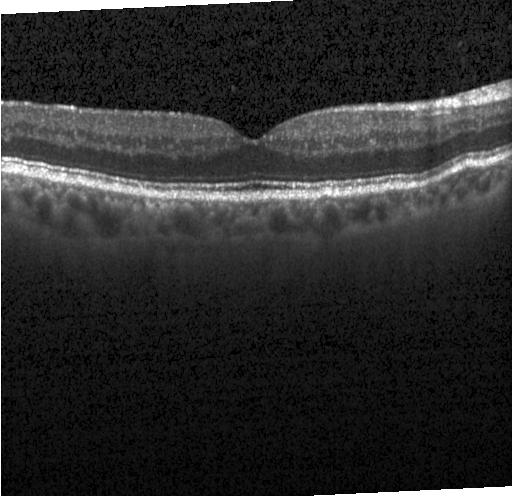

OCT finding: no evidence of CNV, DME, or drusen.